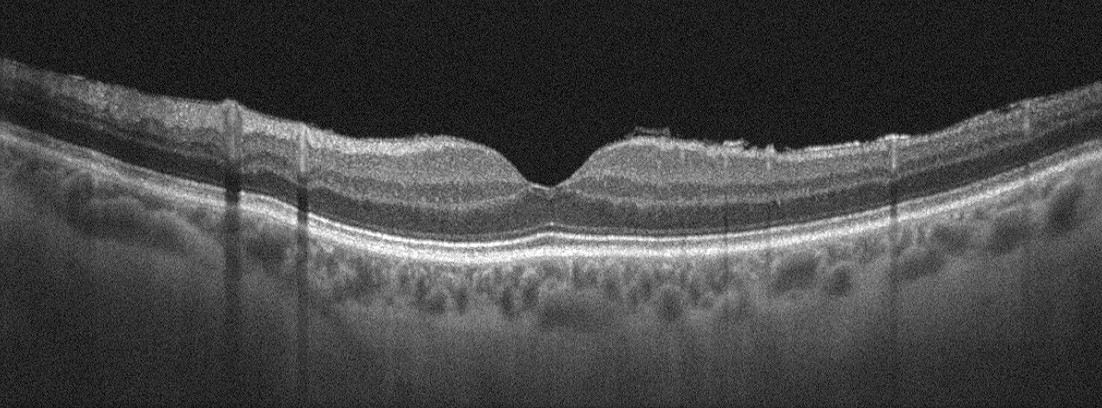 OCT B-scan.
Diagnosis: ERM.